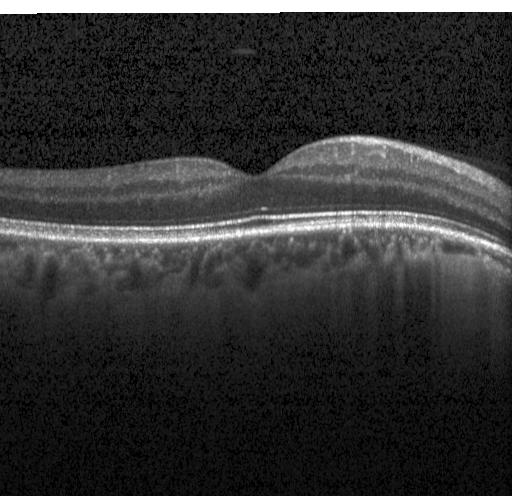 Finding: no choroidal neovascularization, no diabetic macular edema, and no drusen.